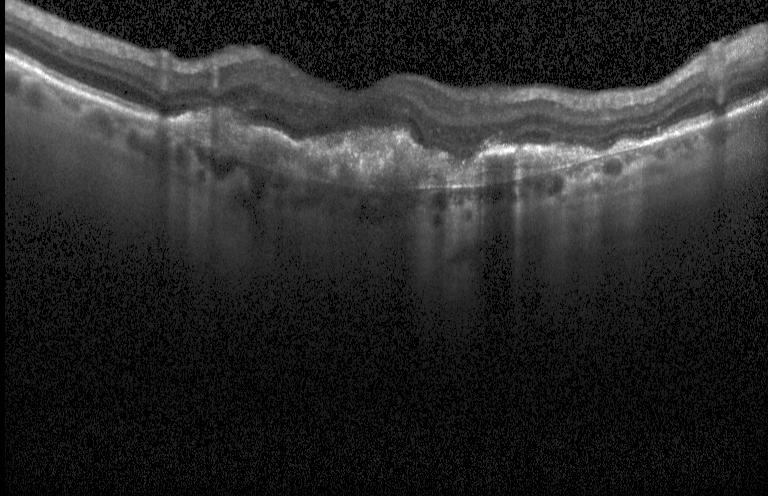 Spectral-domain OCT; optical coherence tomography B-scan — This B-scan demonstrates choroidal neovascularization (CNV).